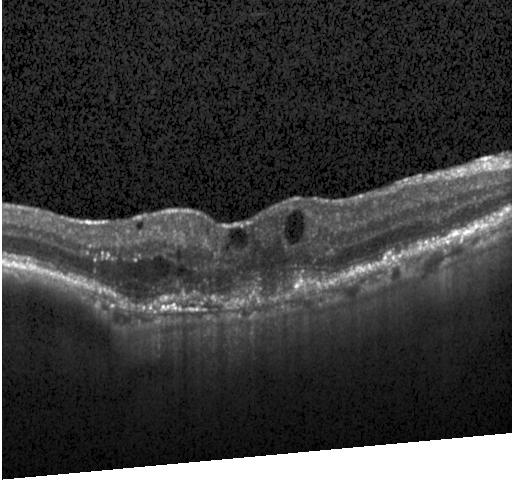 Finding: choroidal neovascularization (CNV).